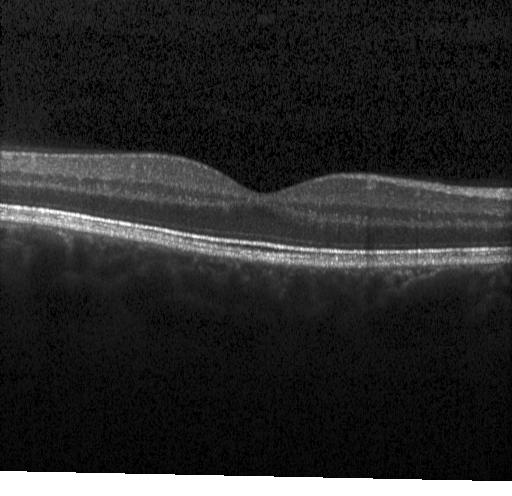 Assessment: no evidence of choroidal neovascularization, diabetic macular edema, or drusen.